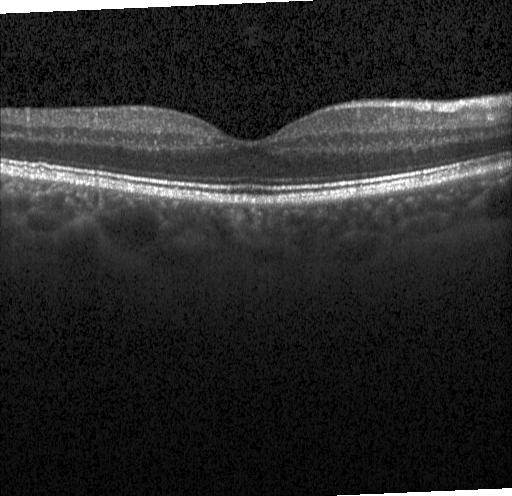

Diagnosis: neither CNV, DME, nor drusen.